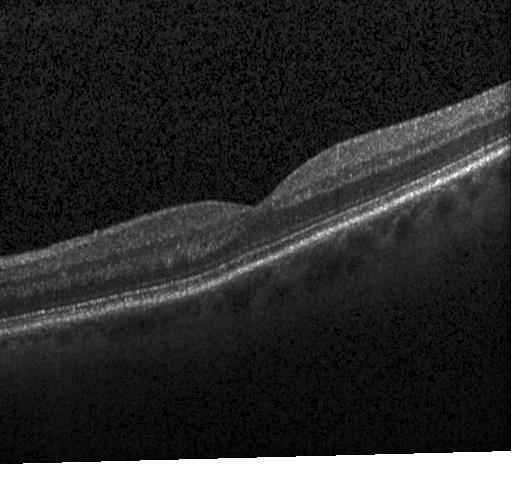
Dx: no choroidal neovascularization, no diabetic macular edema, and no drusen.